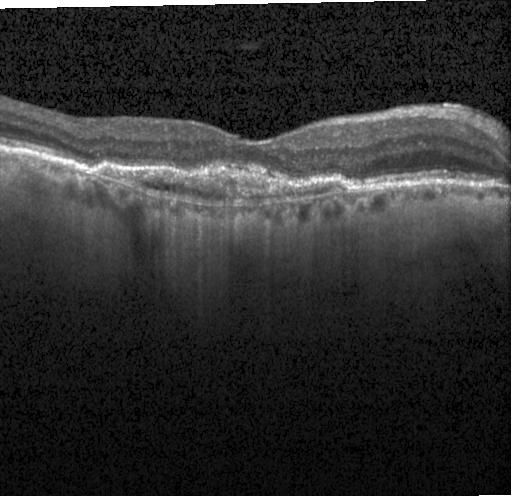
Retinal OCT cross-section; spectral-domain optical coherence tomography
Choroidal neovascularization.